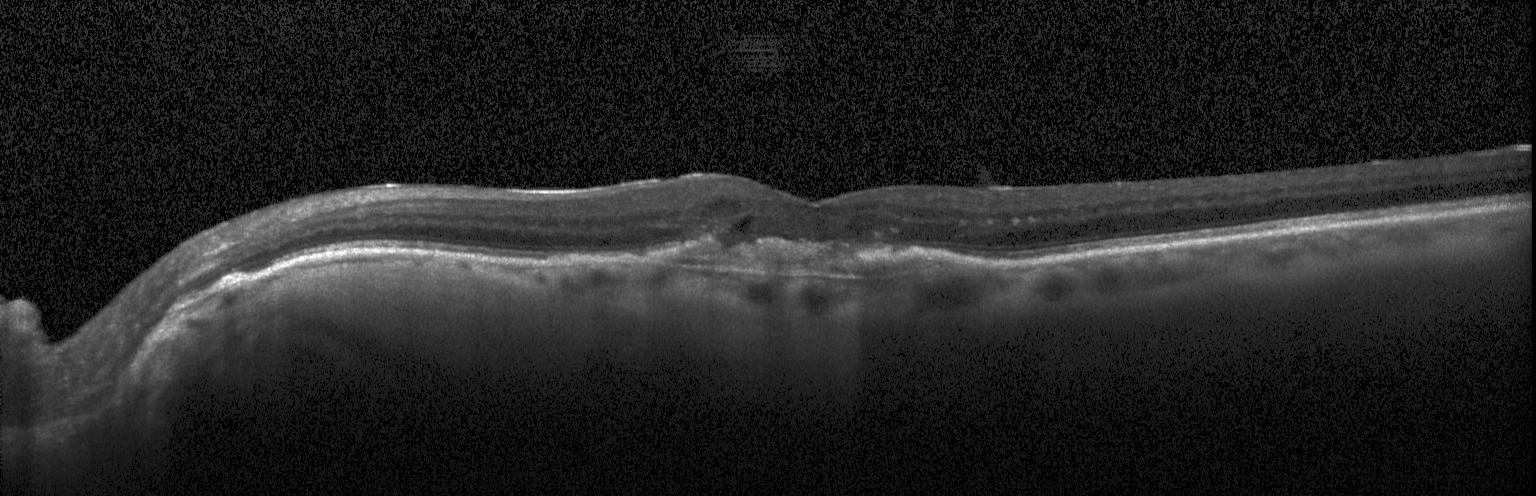

Optical coherence tomography B-scan
Dx: a choroidal neovascular membrane.